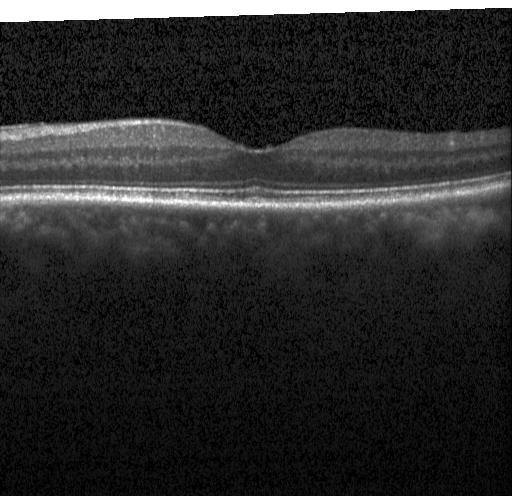
Macular OCT: no evidence of choroidal neovascularization, diabetic macular edema, or drusen.